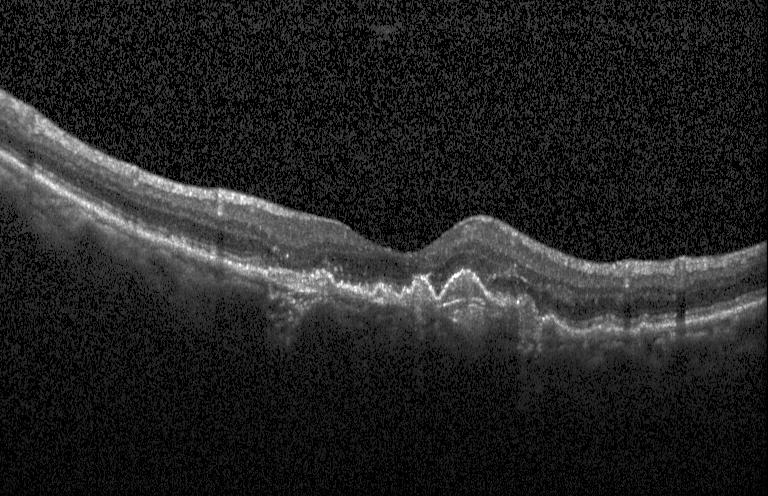
Finding: CNV.